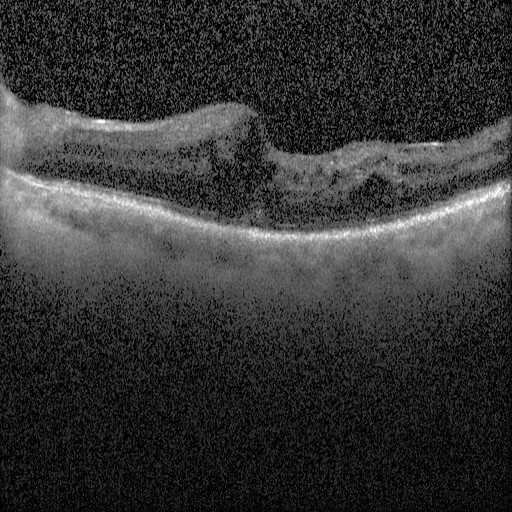
Spectral-domain OCT B-scan: diabetic macular edema (DME).